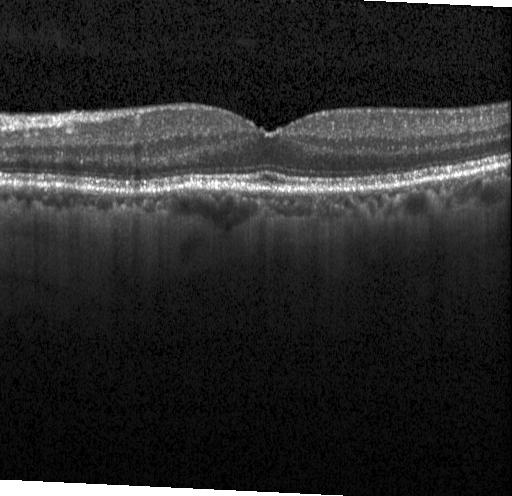
Diagnosis: no CNV, DME, or drusen.